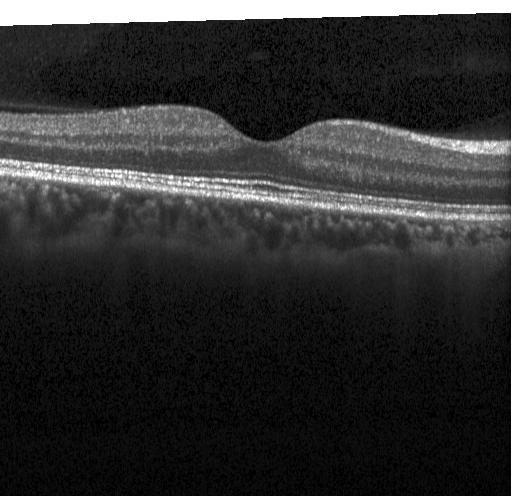

Optical coherence tomography scan — Impression: no choroidal neovascularization, no diabetic macular edema, and no drusen.